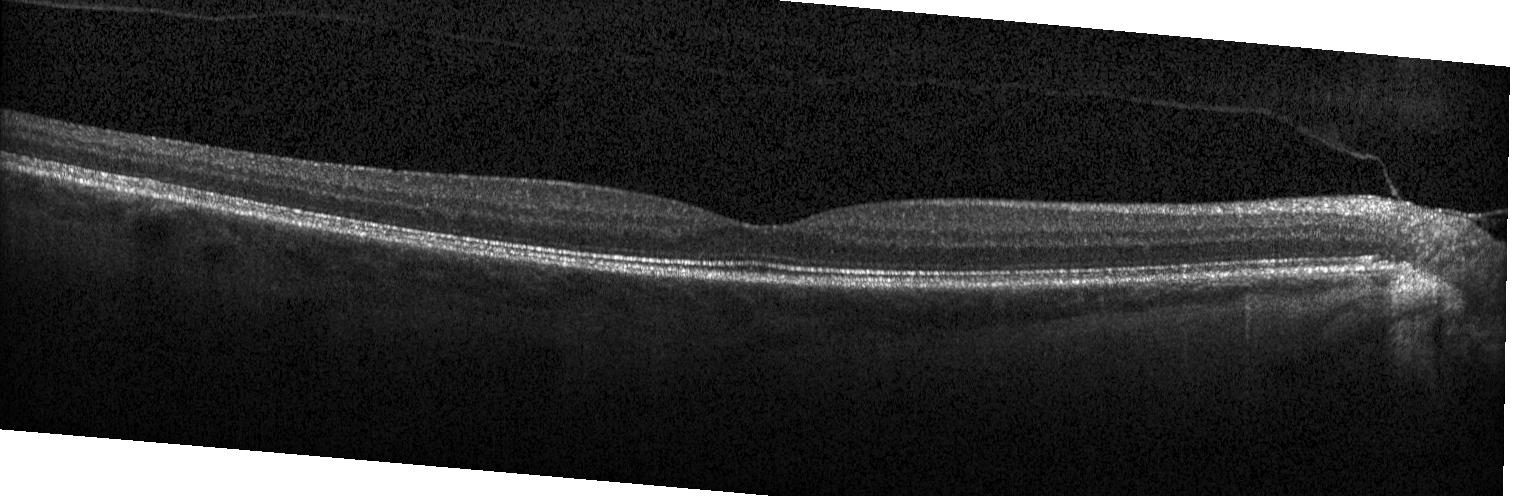 No choroidal neovascularization, no diabetic macular edema, and no drusen.